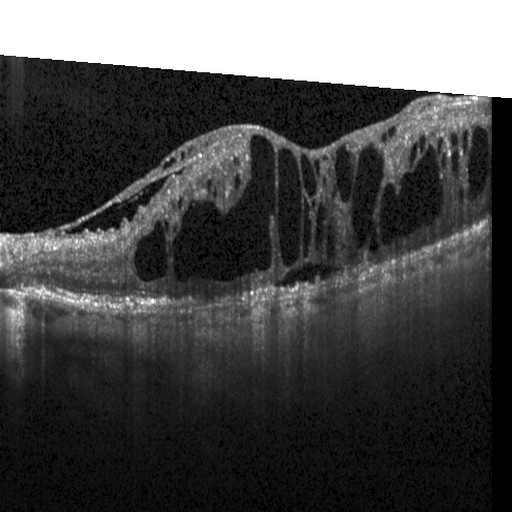 Assessment: DME.